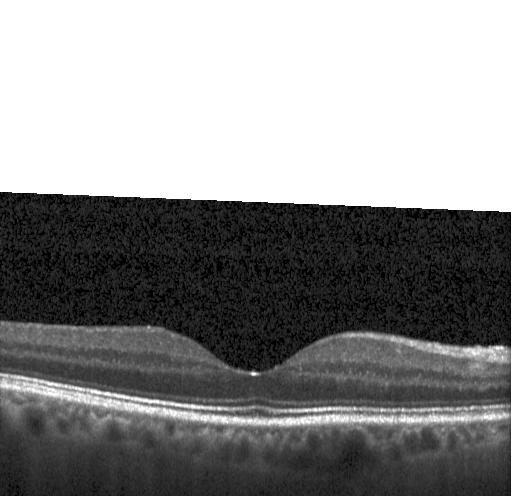

Assessment: no CNV, no DME, and no drusen.